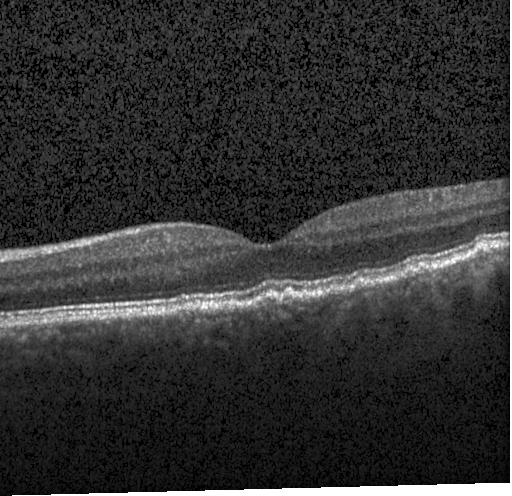 Impression: sub-RPE drusenoid deposits.